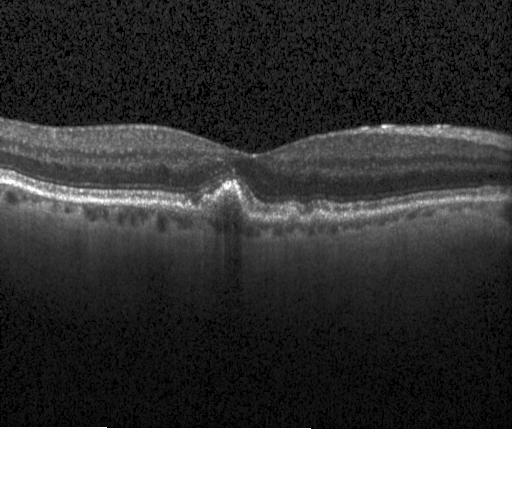

Impression: sub-RPE drusenoid deposits.